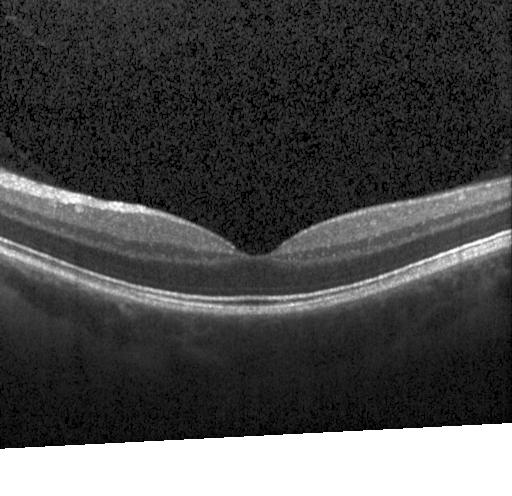 OCT line scan.
This B-scan demonstrates no evidence of CNV, DME, or drusen.